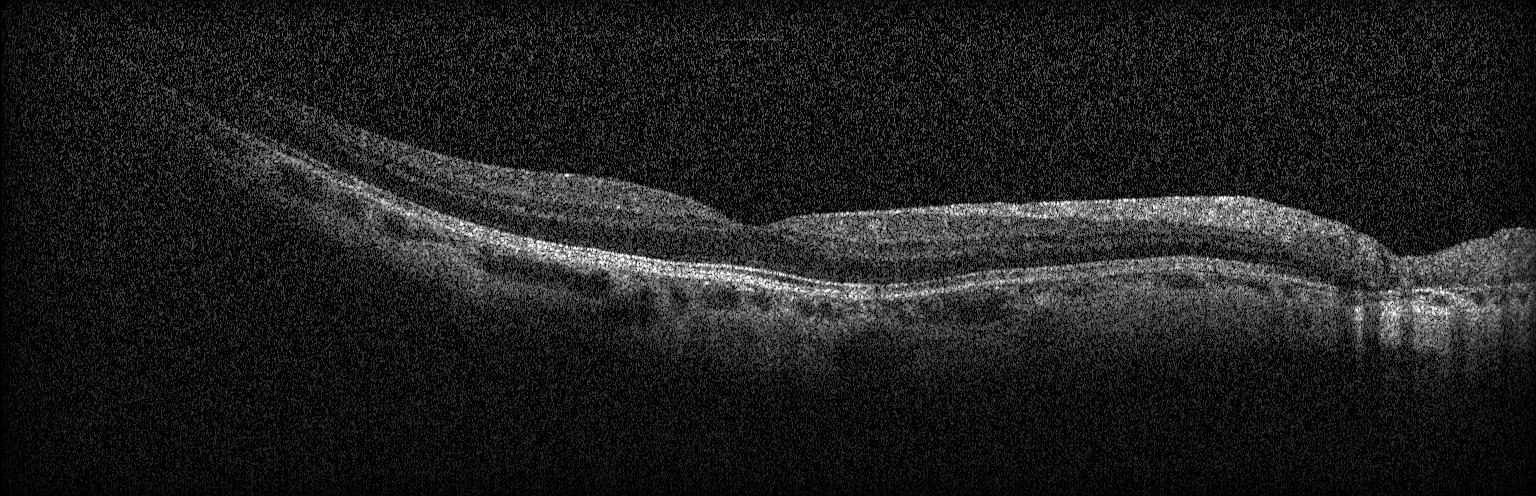
OCT B-scan.
Impression: no choroidal neovascularization, diabetic macular edema, or drusen.